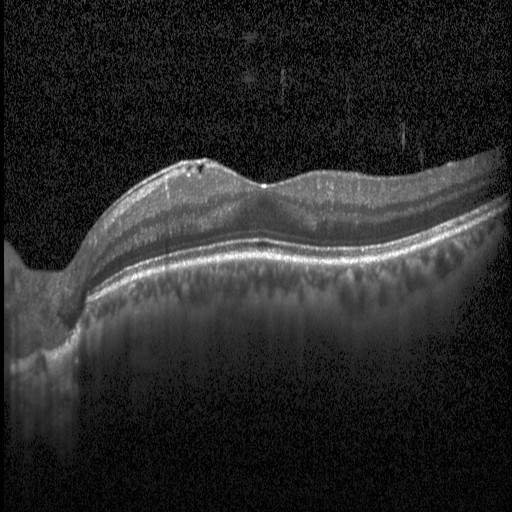
OCT B-scan
Finding: diabetic macular edema (DME).